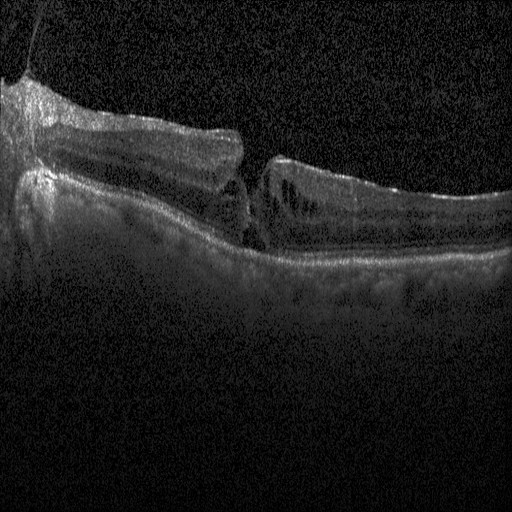
Retinal OCT cross-section. Through the macula. Acquired on a Heidelberg Spectralis.
Diagnosis: diabetic macular edema.